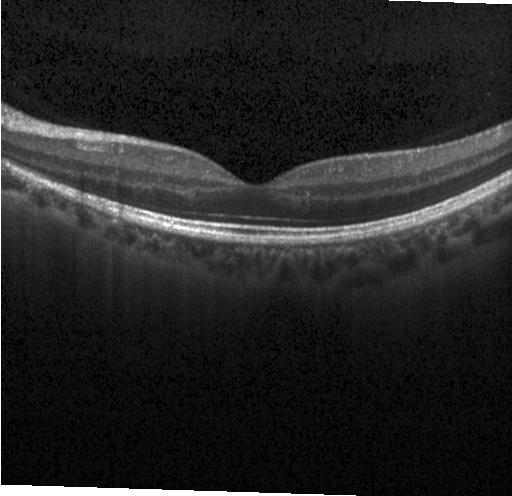
Finding: no evidence of choroidal neovascularization, diabetic macular edema, or drusen.